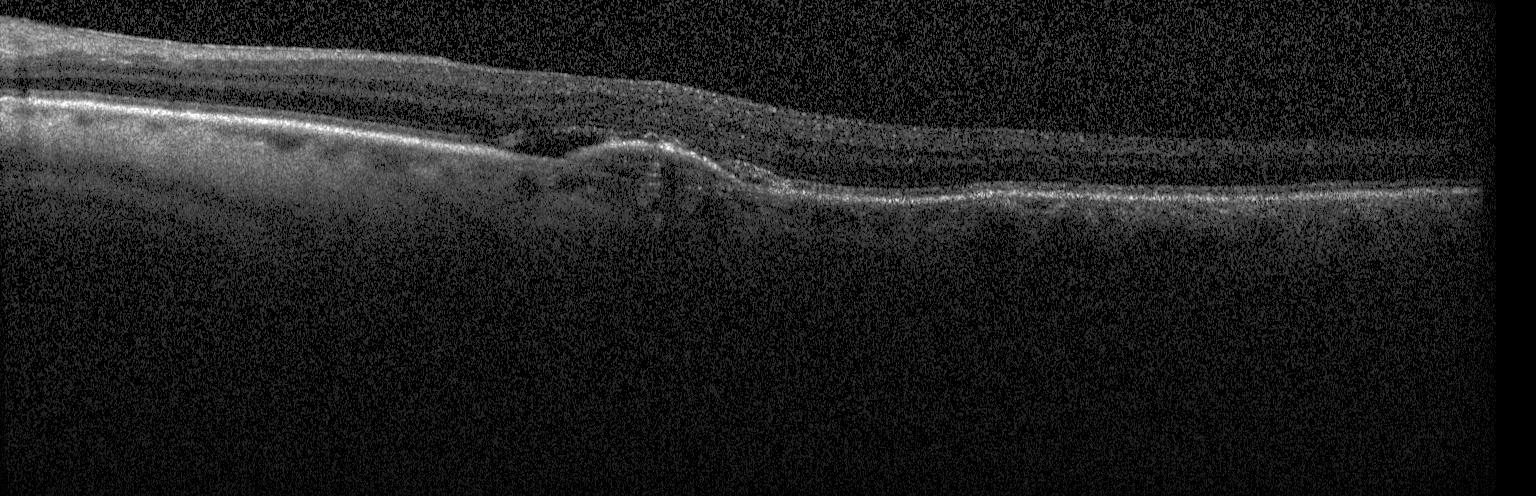

OCT B-scan
Diagnosis: choroidal neovascularization.